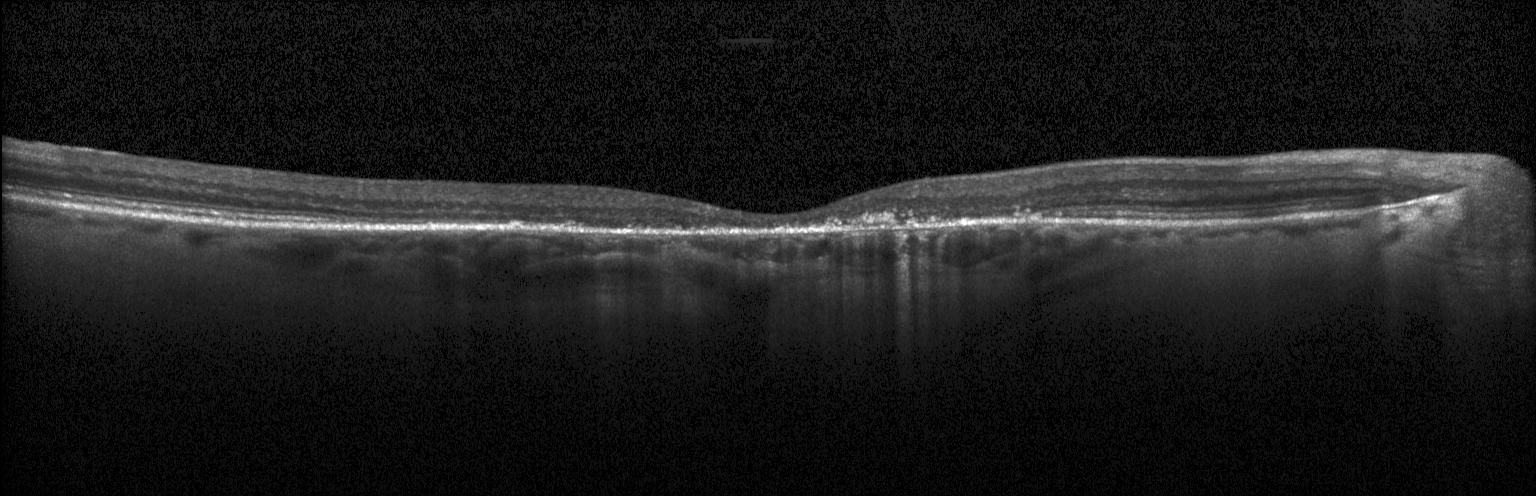
Diagnosis: choroidal neovascularization (CNV).